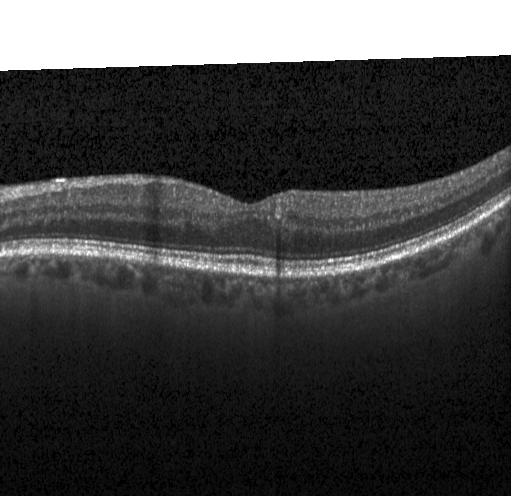
SD-OCT; retinal OCT B-scan; through the macula. Dx: no evidence of CNV, DME, or drusen.